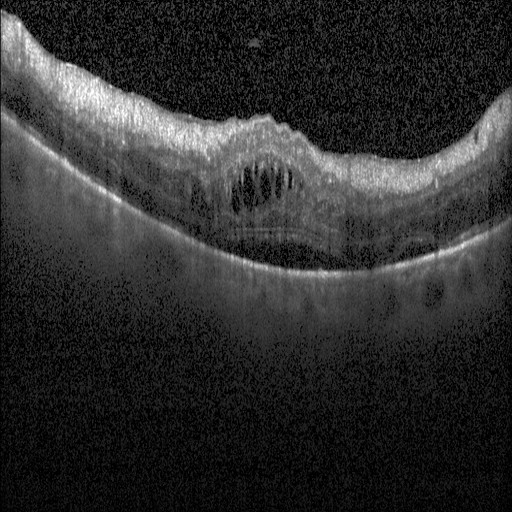
OCT finding: diabetic macular edema (DME).